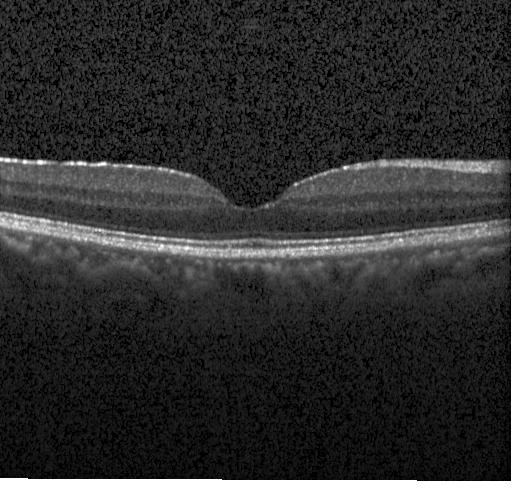

Spectral-domain OCT B-scan: no CNV, DME, or drusen.